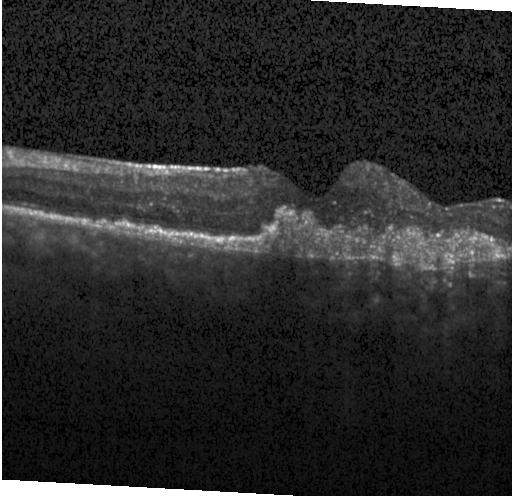
Macular scan; Heidelberg Spectralis; retinal OCT cross-section; spectral-domain OCT — Impression: choroidal neovascularization.